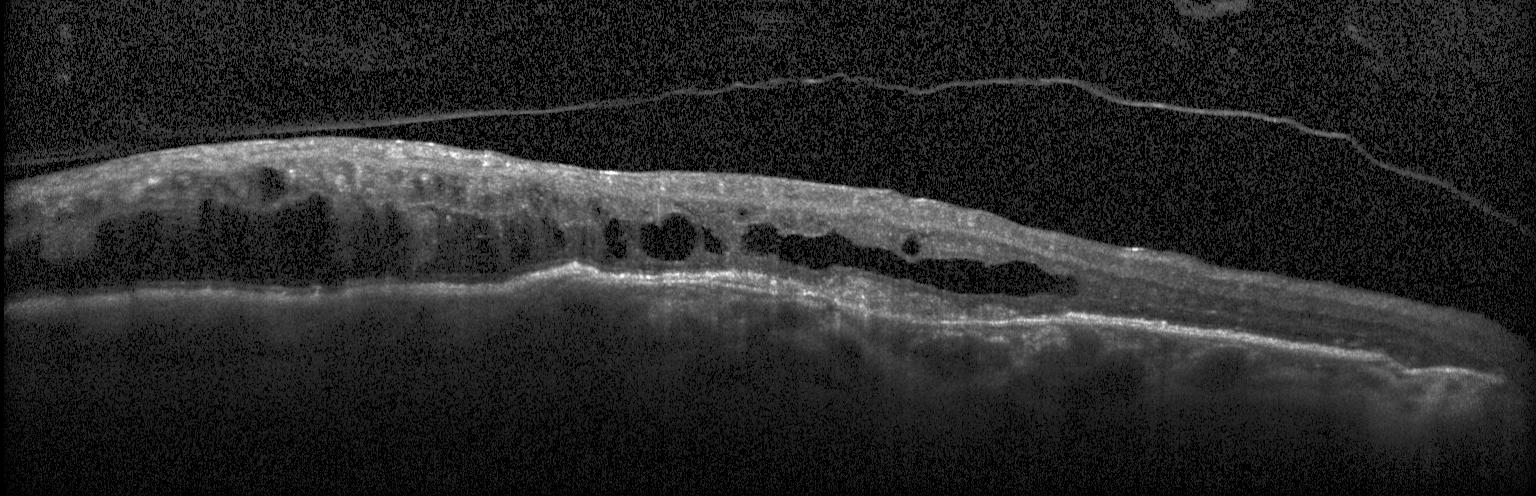

Optical coherence tomography B-scan. Horizontal scan through the fovea. Spectral-domain OCT. Heidelberg Spectralis
Diagnosis: choroidal neovascularization (CNV).